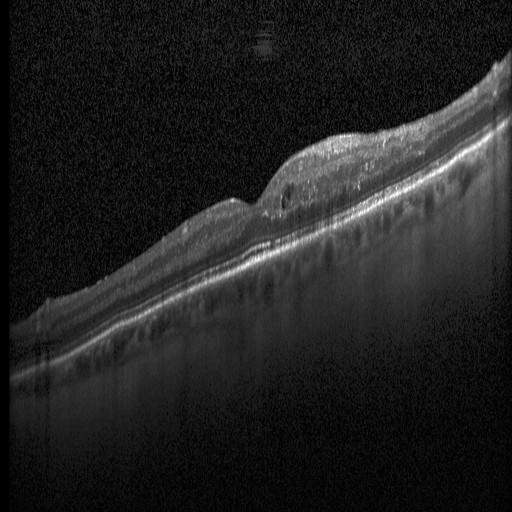 SD-OCT · OCT line scan · Heidelberg Spectralis OCT system · through the macula — Diagnosis: diabetic macular edema (DME).